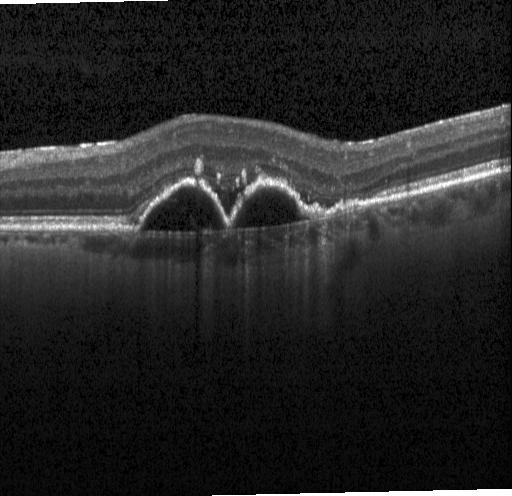 Optical coherence tomography scan. Assessment: a choroidal neovascular membrane.